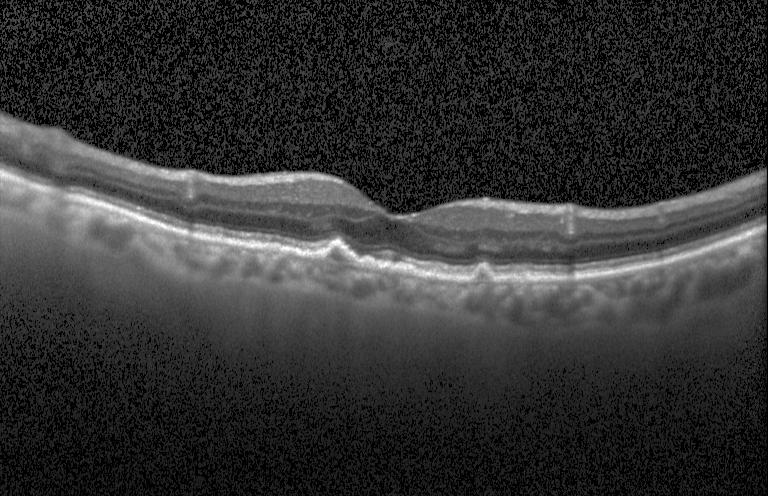

OCT B-scan showing sub-RPE drusenoid deposits.